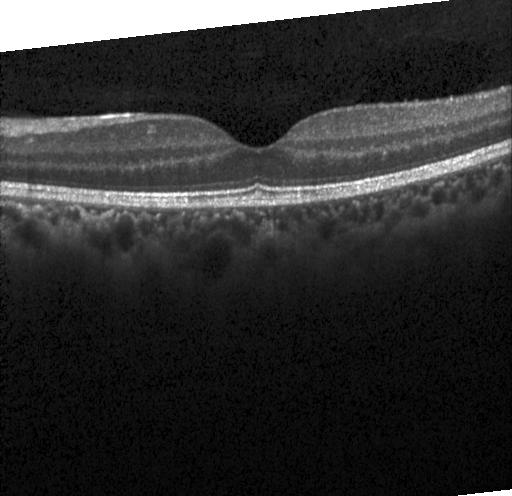

Instrument: Heidelberg Spectralis; optical coherence tomography scan; horizontal scan through the fovea; spectral-domain optical coherence tomography — Assessment: no choroidal neovascularization, no diabetic macular edema, and no drusen.